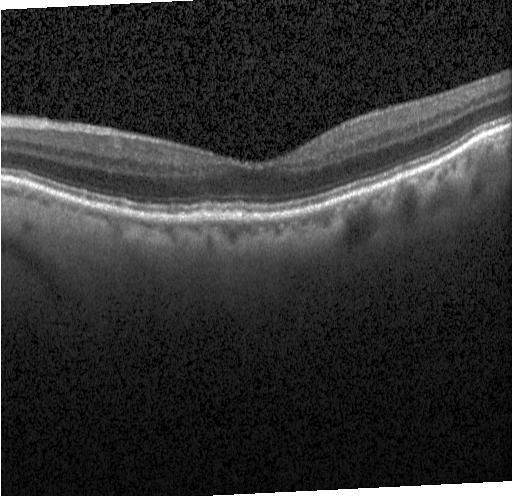
Spectral-domain OCT B-scan: multiple drusen.